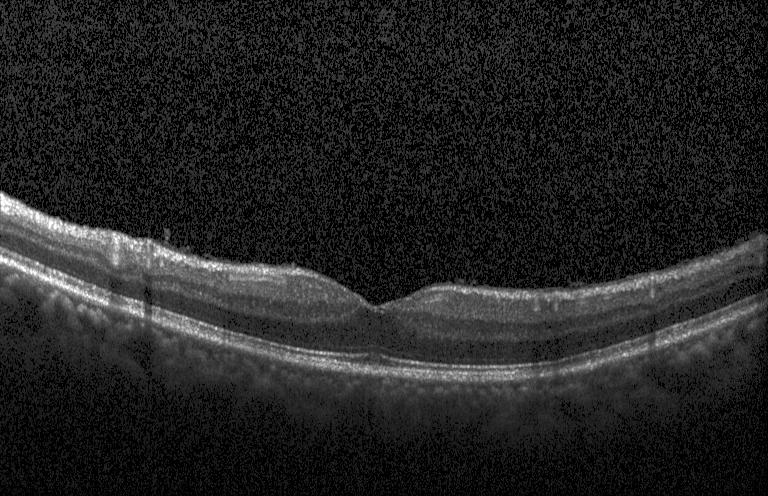 Spectral-domain OCT B-scan: no choroidal neovascularization, no diabetic macular edema, and no drusen.